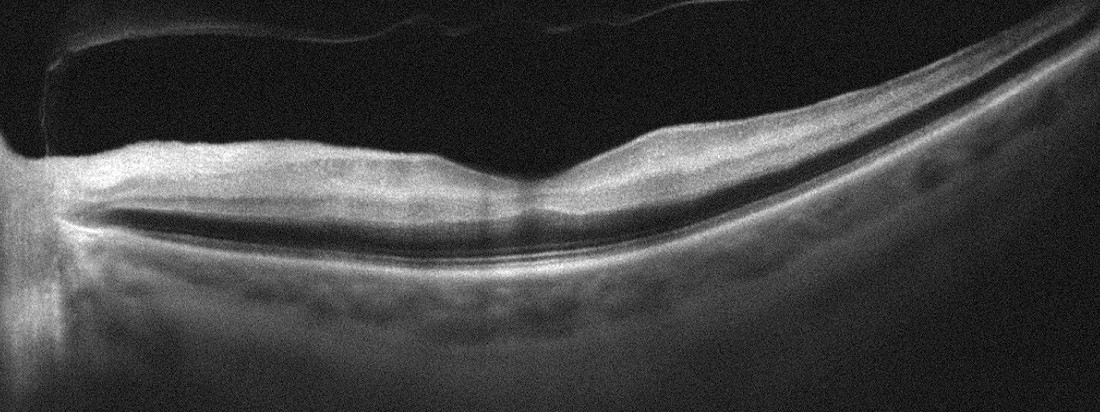

OCT scan showing RAO.